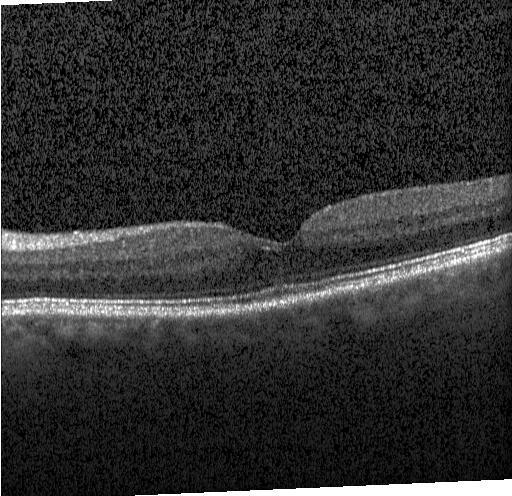

Optical coherence tomography B-scan. The scan shows no choroidal neovascularization, diabetic macular edema, or drusen.